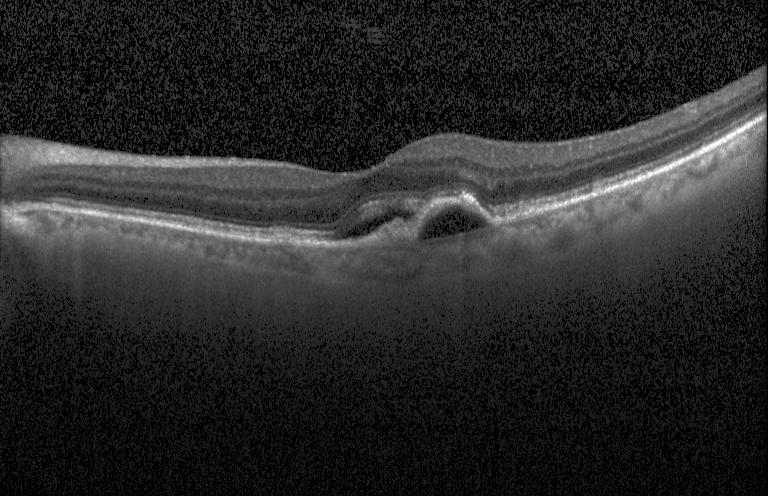
Centered on the fovea · optical coherence tomography scan · Heidelberg Spectralis OCT system · spectral-domain OCT.
Macular OCT: a choroidal neovascular membrane.